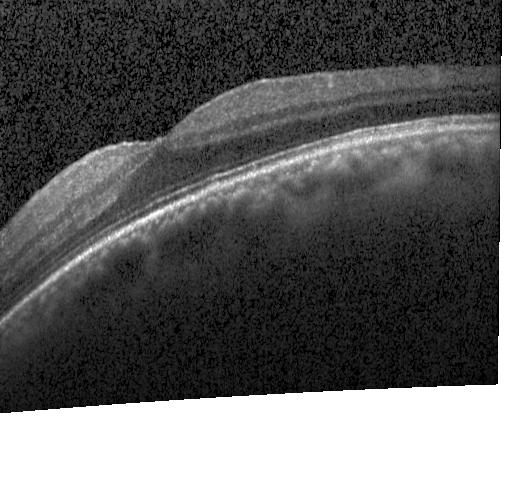 Spectral-domain optical coherence tomography · retinal OCT cross-section · acquired on a Heidelberg Spectralis — Assessment: no choroidal neovascularization, diabetic macular edema, or drusen.